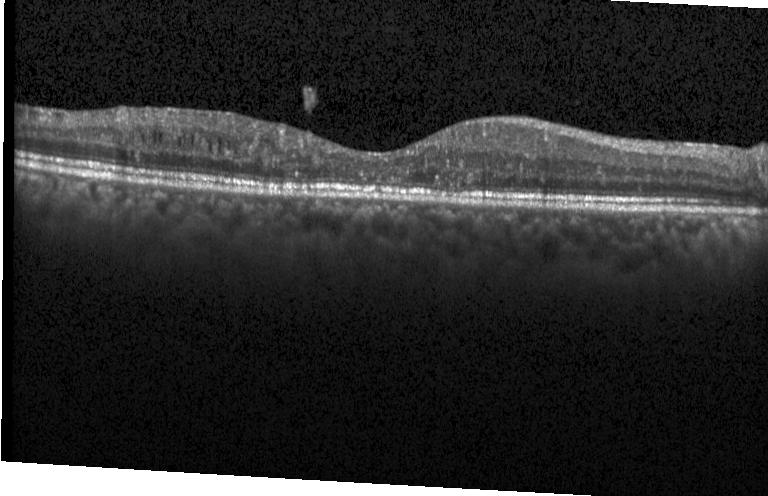 This B-scan demonstrates diabetic macular edema (DME).